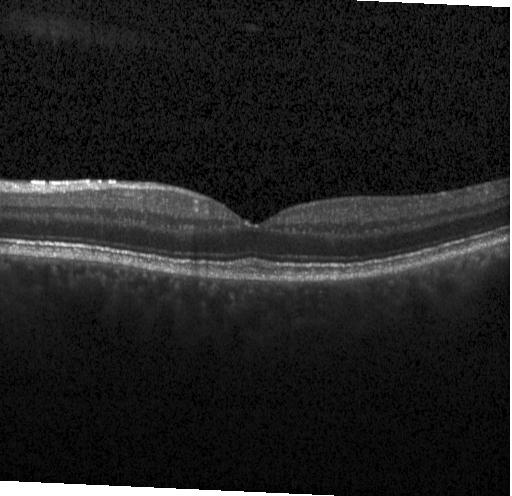 No evidence of CNV, DME, or drusen.